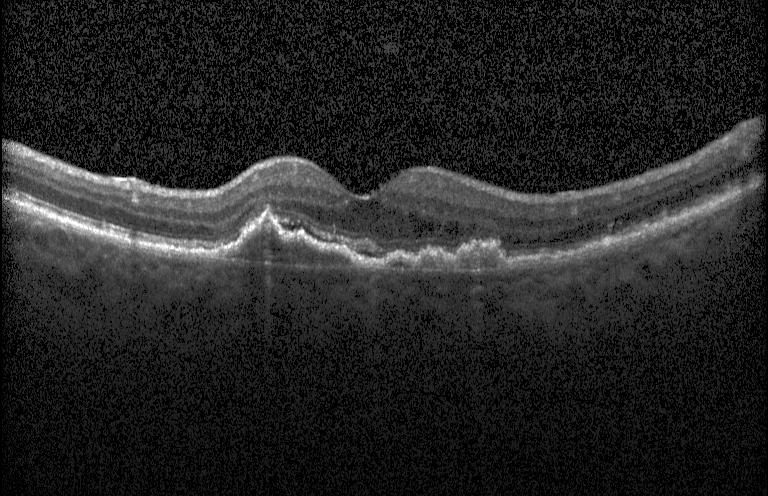 Instrument: Heidelberg Spectralis, fovea-centered, OCT B-scan — OCT finding: a choroidal neovascular membrane.